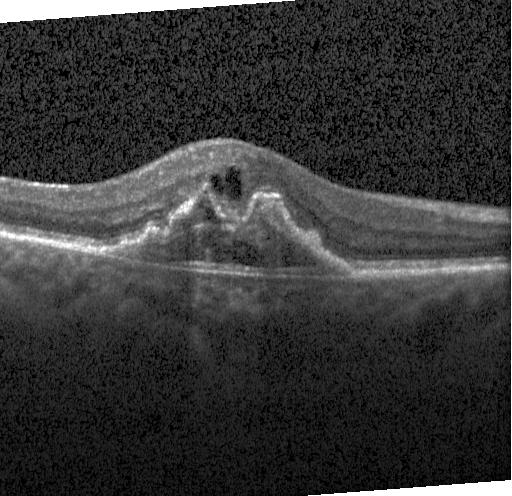
OCT line scan.
Dx: a choroidal neovascular membrane.